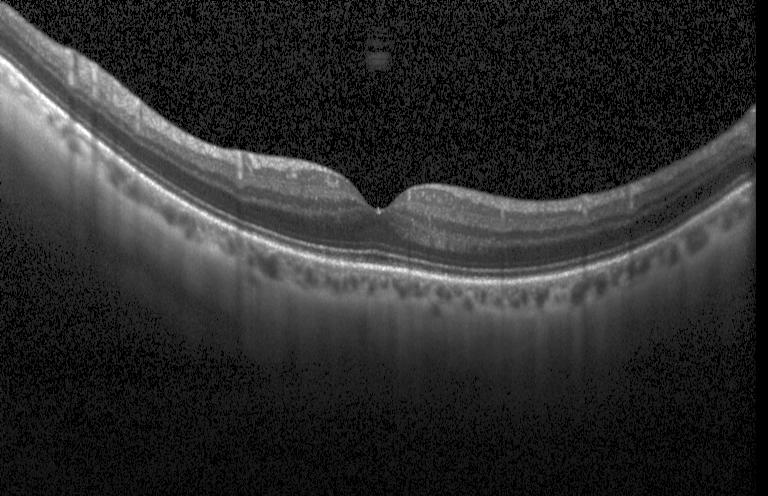

No CNV, no DME, and no drusen.